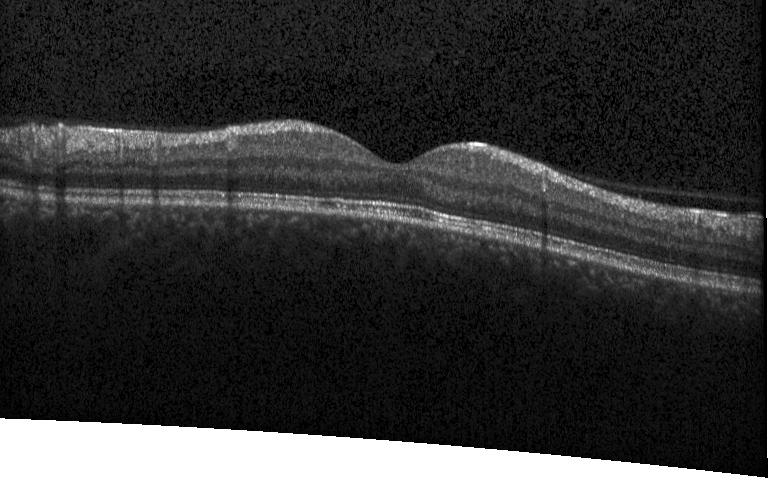
Through the macula, retinal OCT B-scan, spectral-domain optical coherence tomography
Diagnosis: neither choroidal neovascularization, diabetic macular edema, nor drusen.